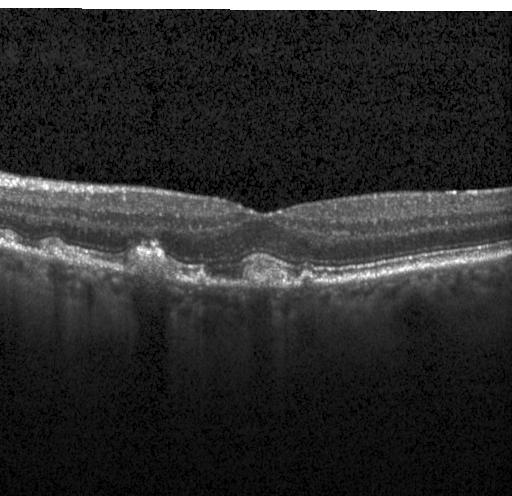

Retinal OCT cross-section. The scan shows CNV.